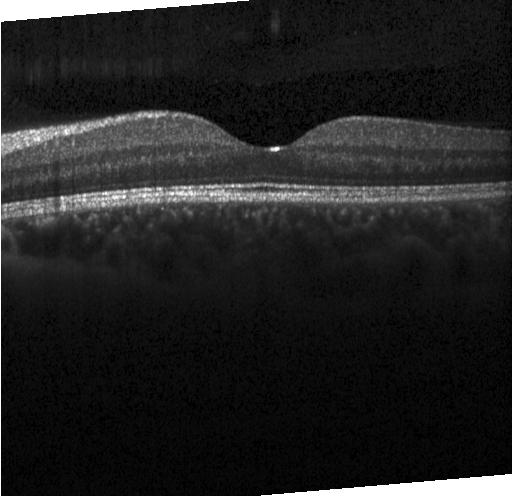
Acquired on a Heidelberg Spectralis · OCT B-scan.
Diagnosis: no CNV, no DME, and no drusen.